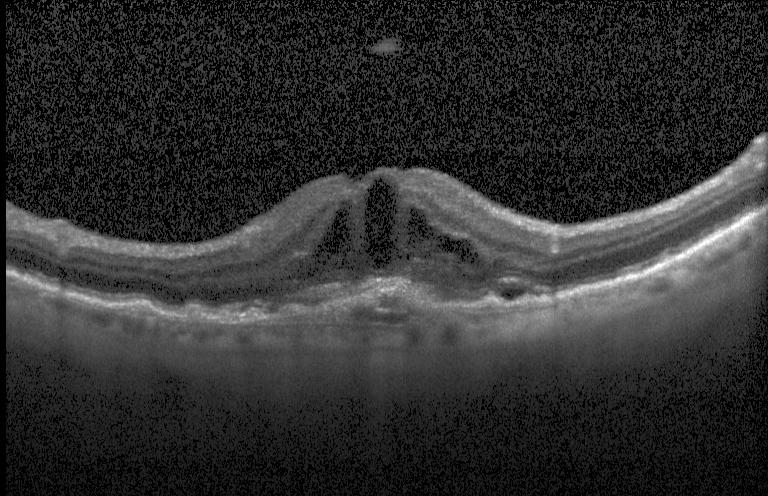 Heidelberg Spectralis OCT system; OCT line scan. Diagnosis: CNV.